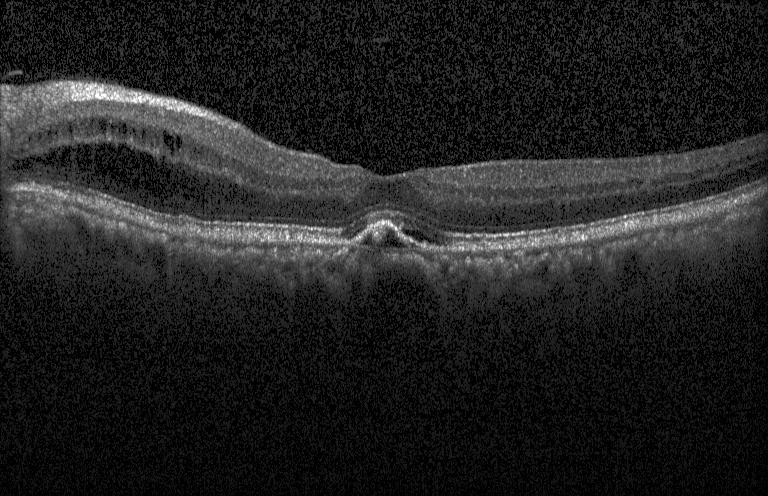
Spectral-domain optical coherence tomography, instrument: Heidelberg Spectralis, optical coherence tomography B-scan, through the macula — Assessment: choroidal neovascularization (CNV).